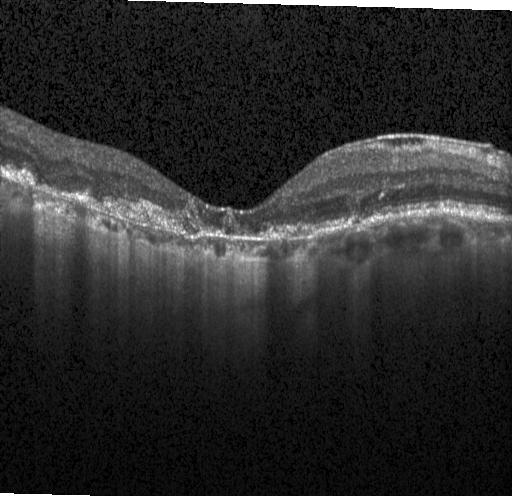

Horizontal scan through the fovea, SD-OCT, OCT line scan, acquired on a Heidelberg Spectralis.
OCT finding: a choroidal neovascular membrane.